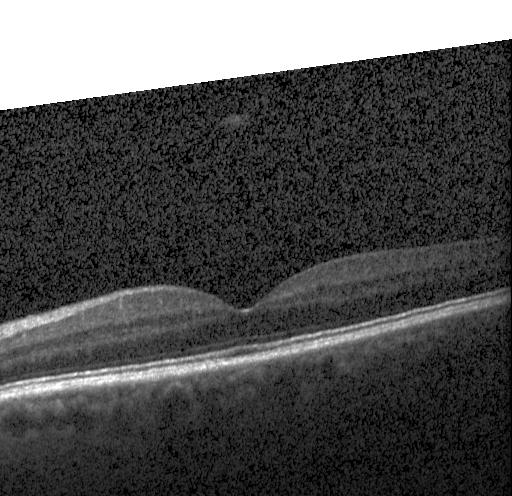
Horizontal scan through the fovea, acquired on a Heidelberg Spectralis, OCT B-scan, SD-OCT
This B-scan demonstrates no evidence of choroidal neovascularization, diabetic macular edema, or drusen.